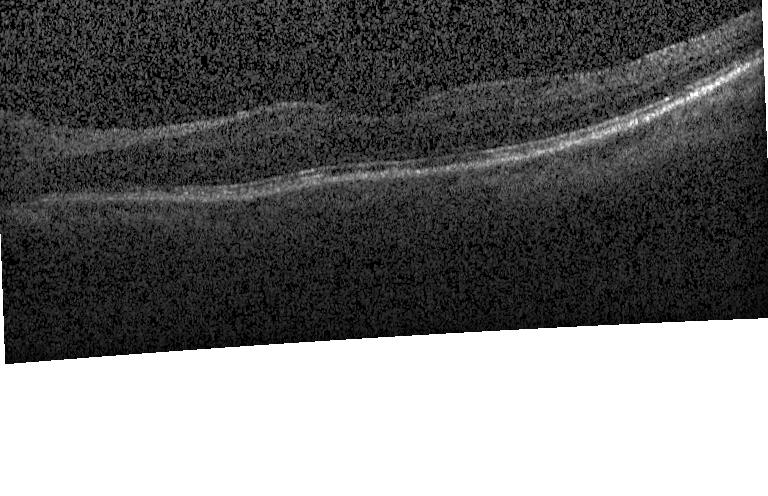

Spectral-domain optical coherence tomography; instrument: Heidelberg Spectralis; optical coherence tomography B-scan; fovea-centered
This B-scan demonstrates no choroidal neovascularization, diabetic macular edema, or drusen.